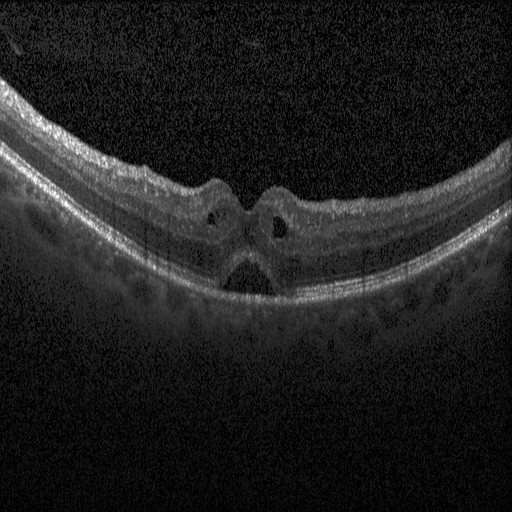 Retinal OCT cross-section, macular scan, spectral-domain optical coherence tomography.
This B-scan demonstrates diabetic macular edema.